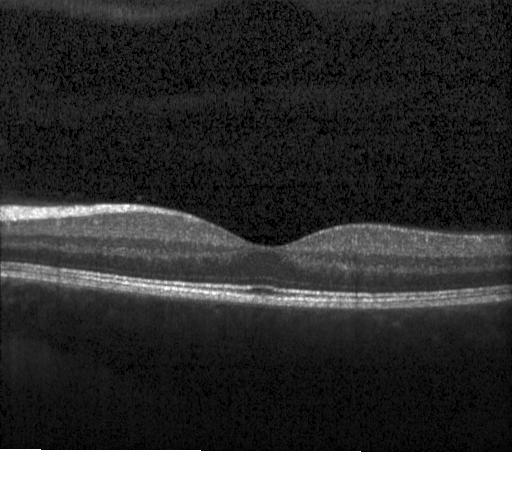 Assessment: no CNV, DME, or drusen.